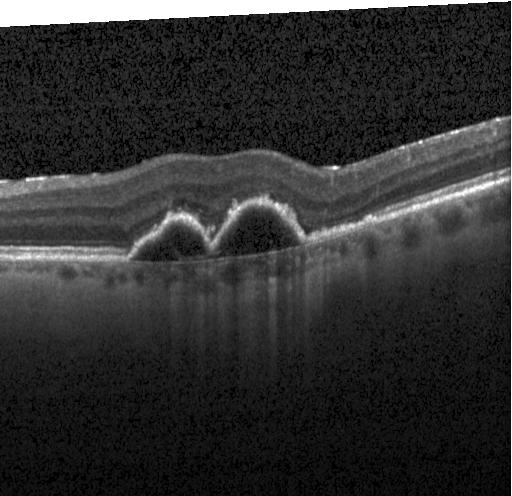 Optical coherence tomography scan.
Impression: choroidal neovascularization.